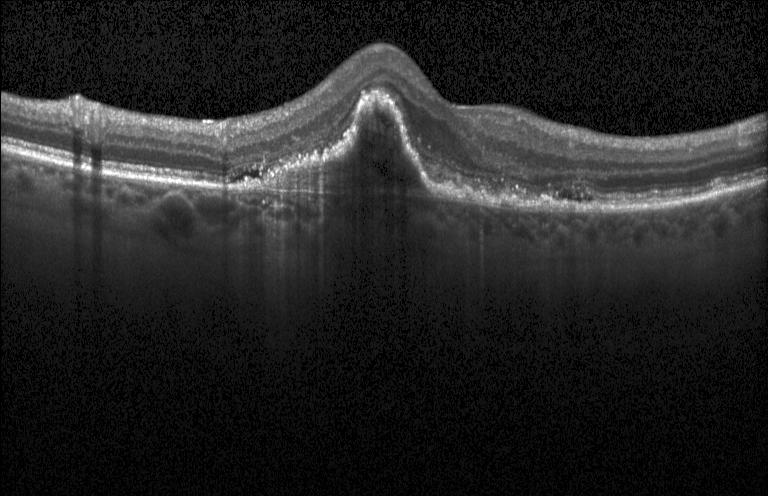 Retinal OCT cross-section
The scan shows a choroidal neovascular membrane.